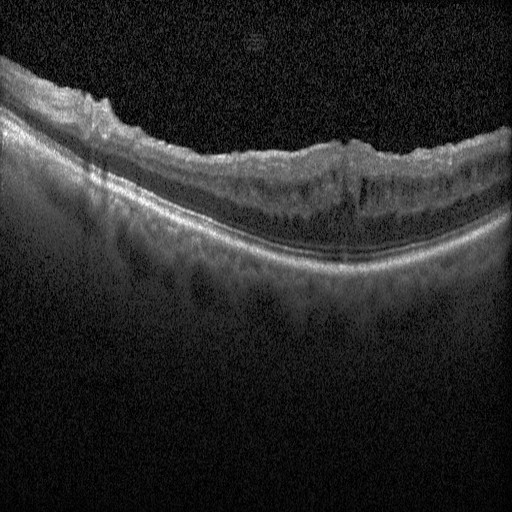 Horizontal scan through the fovea, optical coherence tomography B-scan.
Assessment: DME.